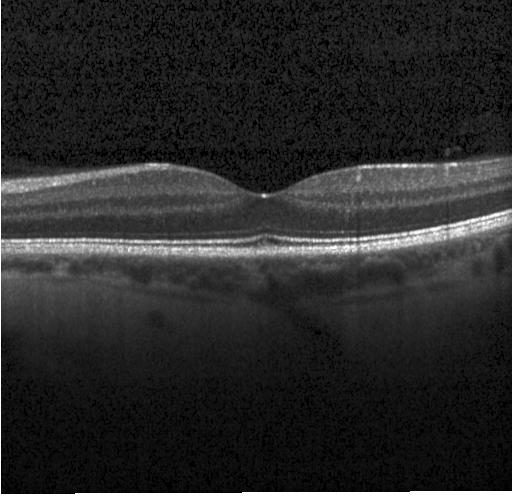 Finding: no choroidal neovascularization, diabetic macular edema, or drusen.